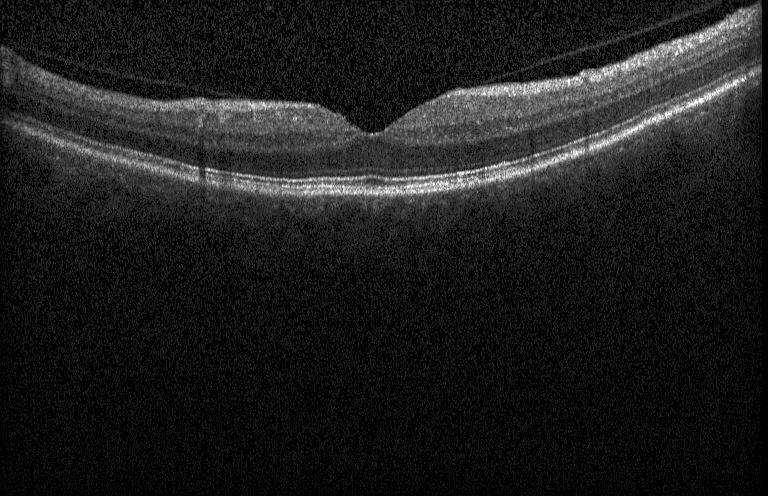

Heidelberg Spectralis, optical coherence tomography B-scan
Impression: no CNV, no DME, and no drusen.